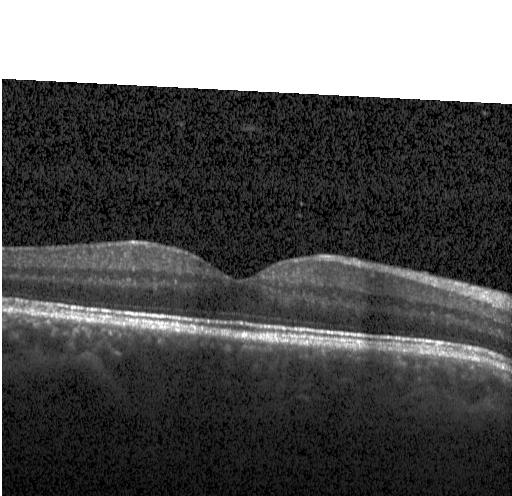 Diagnosis: neither choroidal neovascularization, diabetic macular edema, nor drusen.